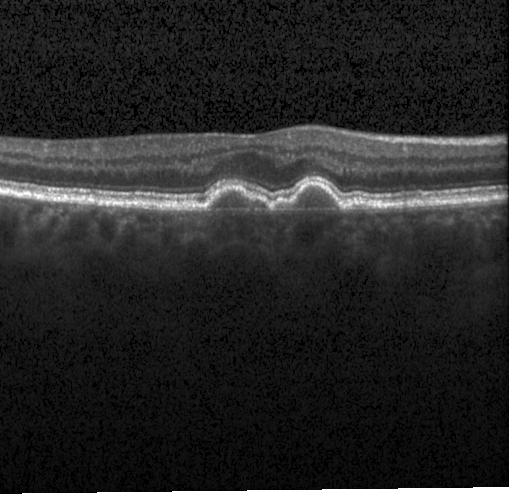 Heidelberg Spectralis · retinal OCT B-scan.
Drusen.